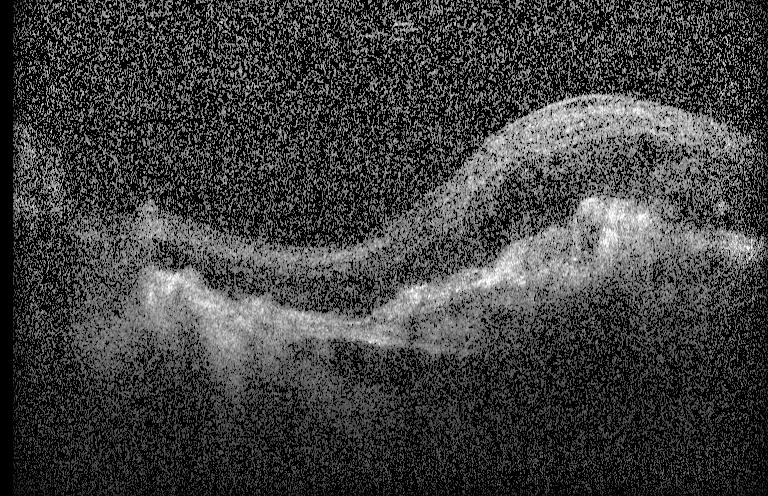

Heidelberg Spectralis. OCT line scan. Spectral-domain OCT. Horizontal scan through the fovea.
Assessment: a choroidal neovascular membrane.